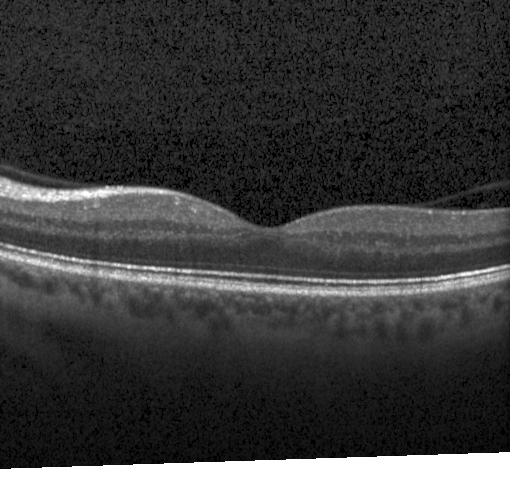

Finding: no evidence of choroidal neovascularization, diabetic macular edema, or drusen.